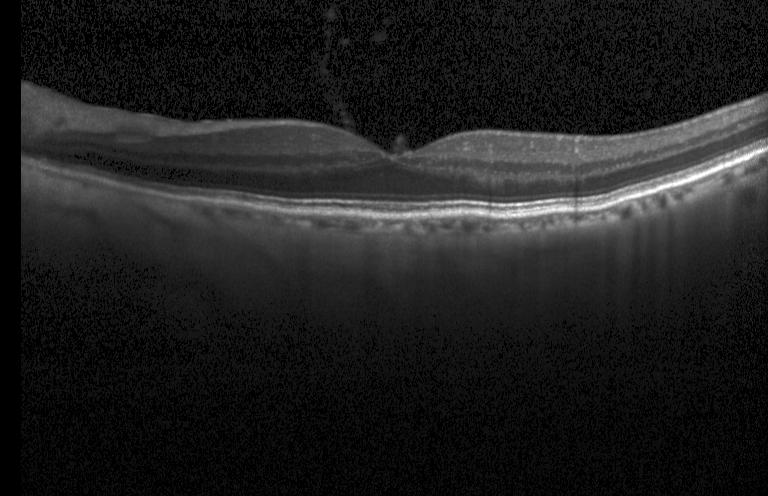 Retinal OCT B-scan — OCT finding: no choroidal neovascularization, diabetic macular edema, or drusen.